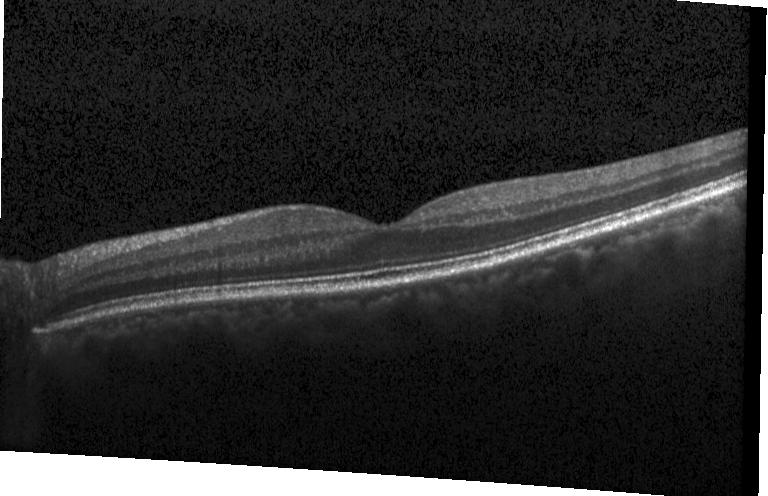 Fovea-centered, optical coherence tomography scan, spectral-domain optical coherence tomography.
Dx: no choroidal neovascularization, no diabetic macular edema, and no drusen.